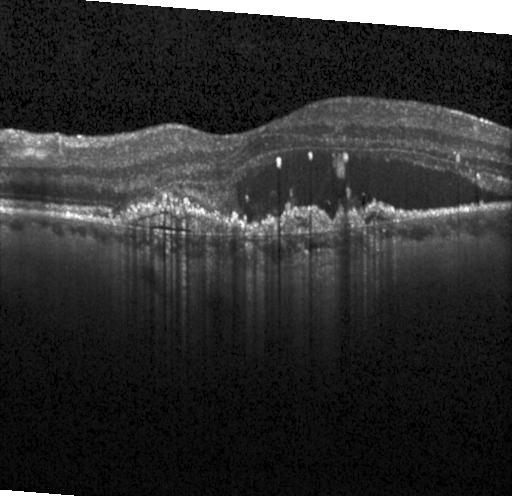
Centered on the fovea · Heidelberg Spectralis OCT system · OCT line scan · spectral-domain optical coherence tomography — Diagnosis: choroidal neovascularization (CNV).